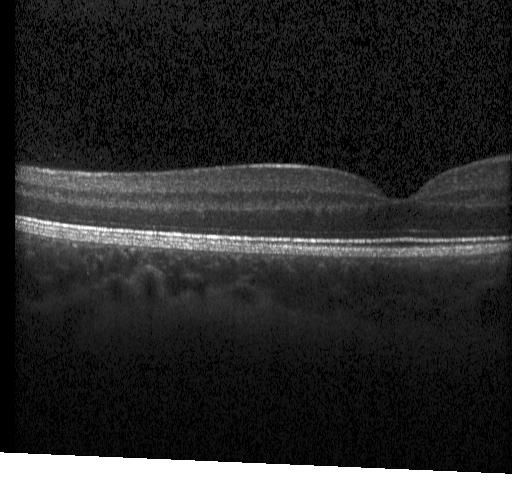 Diagnosis: no CNV, no DME, and no drusen.